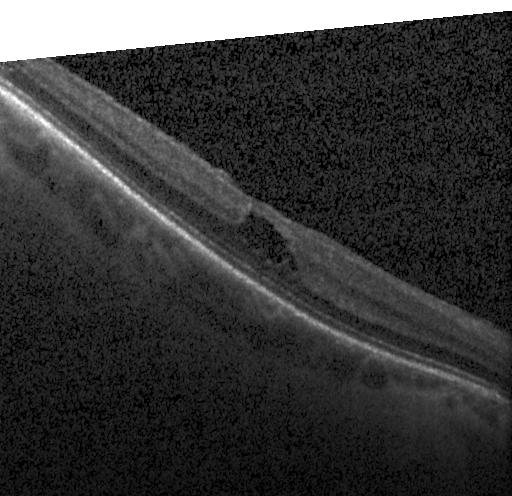
Horizontal scan through the fovea. Spectral-domain optical coherence tomography. Acquired on a Heidelberg Spectralis. OCT B-scan.
Diagnosis: diabetic macular edema (DME).